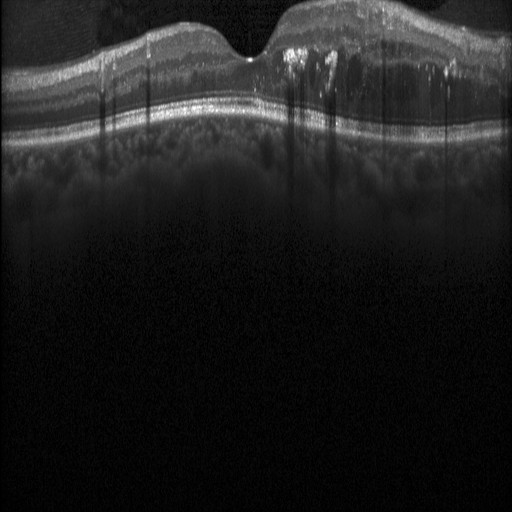 Spectral-domain OCT · horizontal scan through the fovea · OCT line scan · acquired on a Heidelberg Spectralis
Finding: diabetic macular edema.